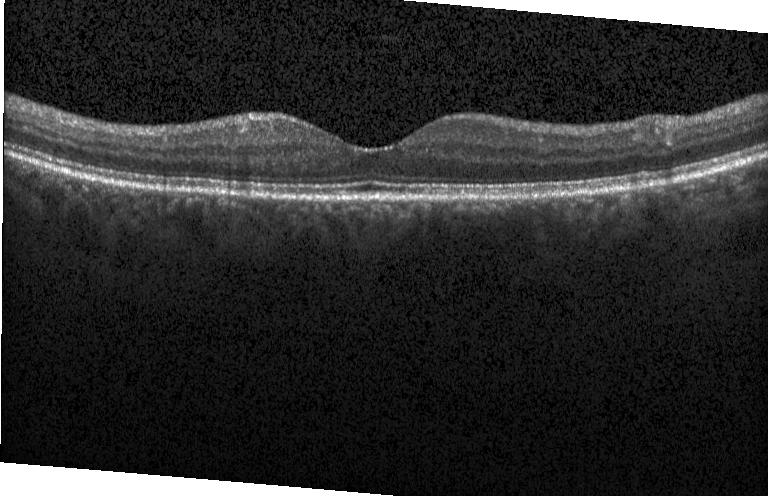 Optical coherence tomography B-scan. Spectral-domain OCT. Macular scan. Heidelberg Spectralis
Diagnosis: no evidence of choroidal neovascularization, diabetic macular edema, or drusen.